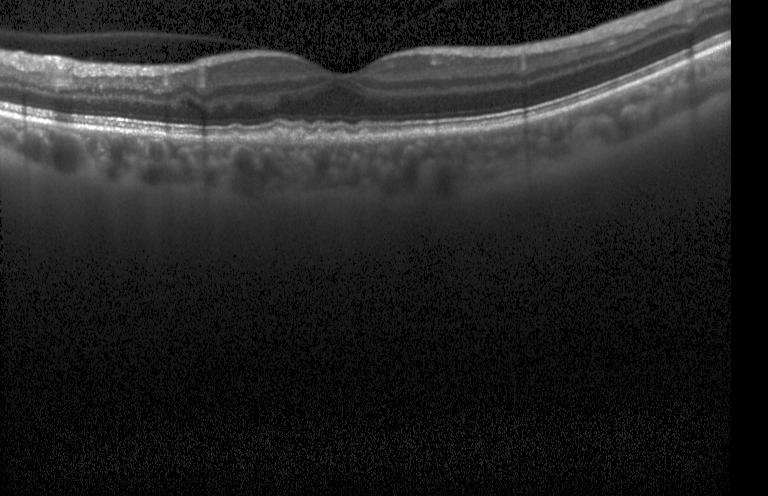
Spectral-domain optical coherence tomography, fovea-centered, acquired on a Heidelberg Spectralis, optical coherence tomography B-scan. Finding: sub-RPE drusenoid deposits.